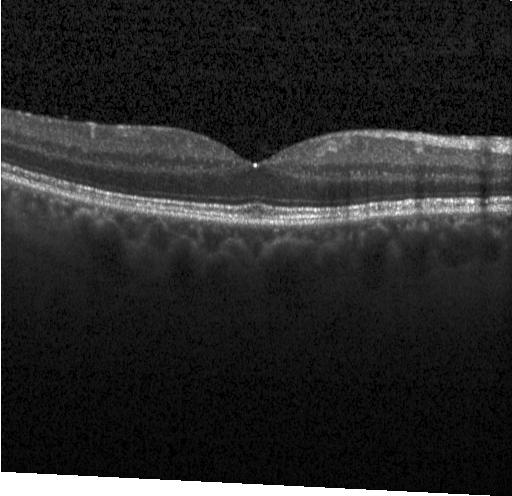
Spectral-domain optical coherence tomography · retinal OCT cross-section — OCT finding: no evidence of CNV, DME, or drusen.